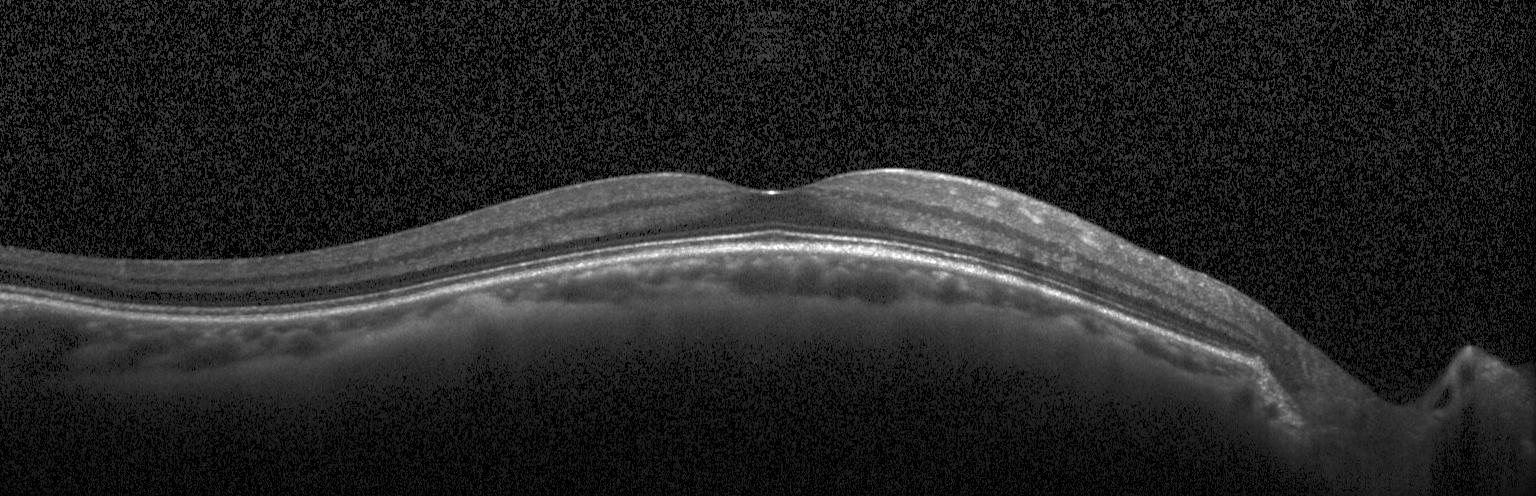
Through the macula; OCT B-scan; Heidelberg Spectralis OCT system
This B-scan demonstrates neither choroidal neovascularization, diabetic macular edema, nor drusen.